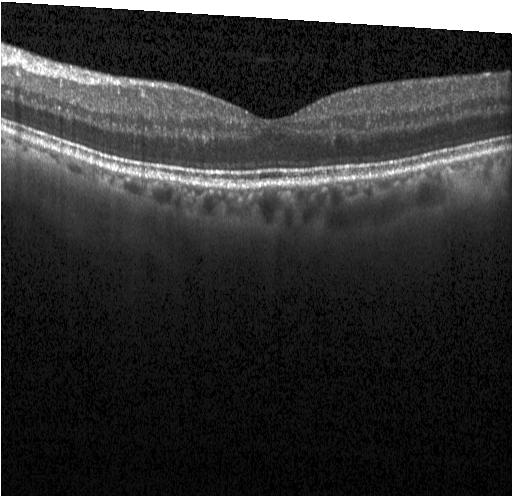
Diagnosis: no choroidal neovascularization, diabetic macular edema, or drusen.